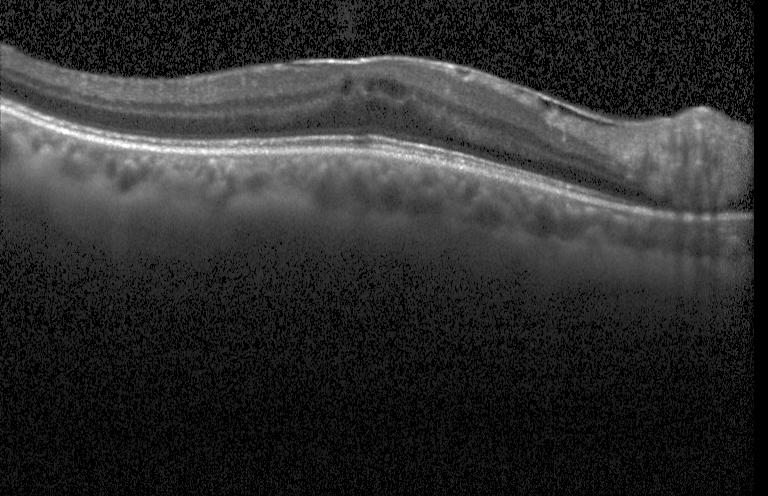
Retinal OCT cross-section showing DME.